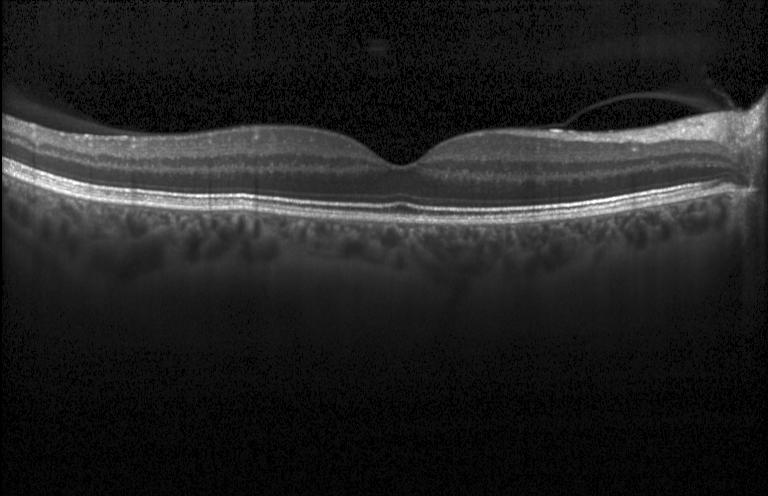 Optical coherence tomography scan; acquired on a Heidelberg Spectralis; spectral-domain OCT.
Diagnosis: no evidence of choroidal neovascularization, diabetic macular edema, or drusen.